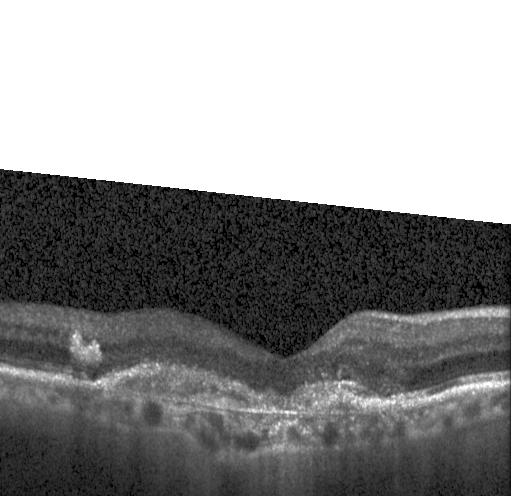 Impression: a choroidal neovascular membrane.